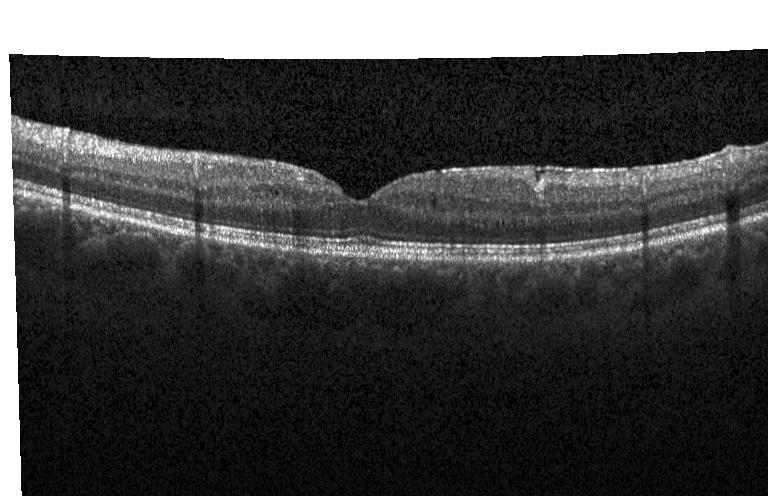

OCT B-scan. Fovea-centered.
Impression: diabetic macular edema (DME).